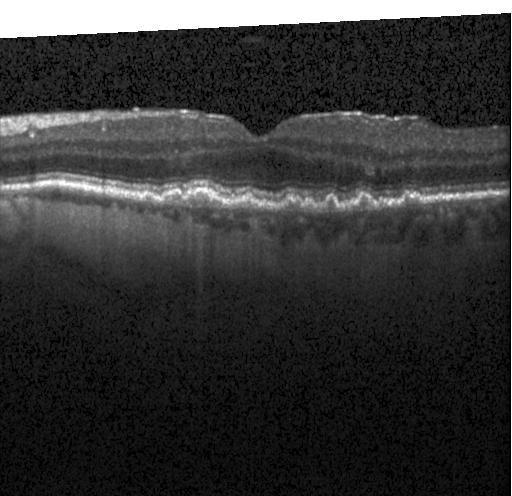 Dx: multiple drusen.